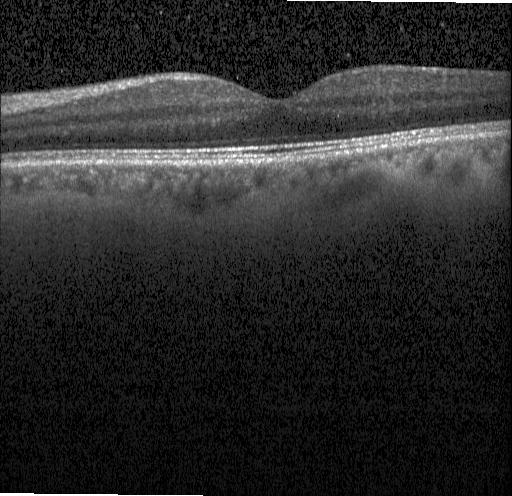

OCT line scan · spectral-domain optical coherence tomography · instrument: Heidelberg Spectralis — No choroidal neovascularization, no diabetic macular edema, and no drusen.